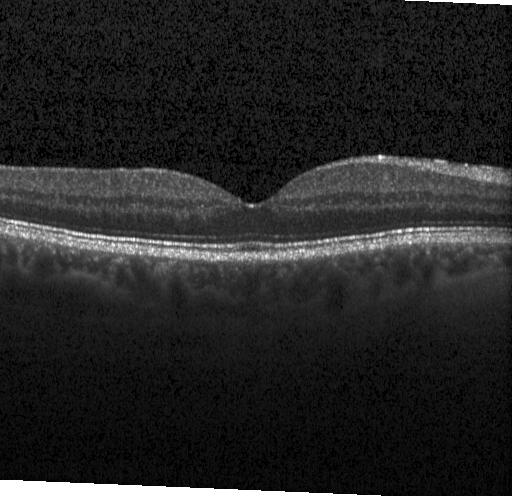
Heidelberg Spectralis OCT system · retinal OCT cross-section.
Finding: no evidence of choroidal neovascularization, diabetic macular edema, or drusen.